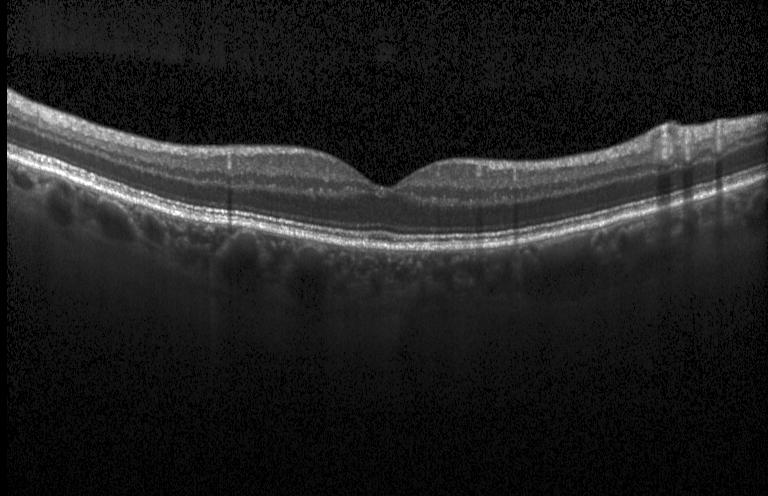

Retinal OCT B-scan · spectral-domain OCT · macular scan — Diagnosis: no choroidal neovascularization, no diabetic macular edema, and no drusen.